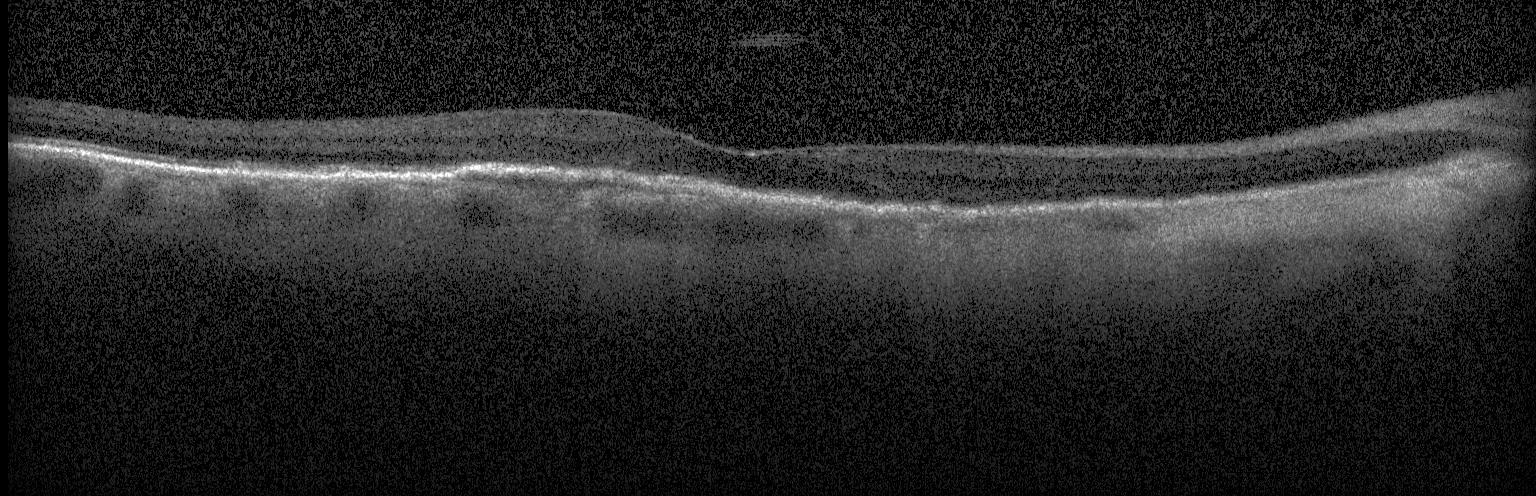
Retinal OCT B-scan. Macular scan. Instrument: Heidelberg Spectralis. Spectral-domain optical coherence tomography
Assessment: choroidal neovascularization (CNV).